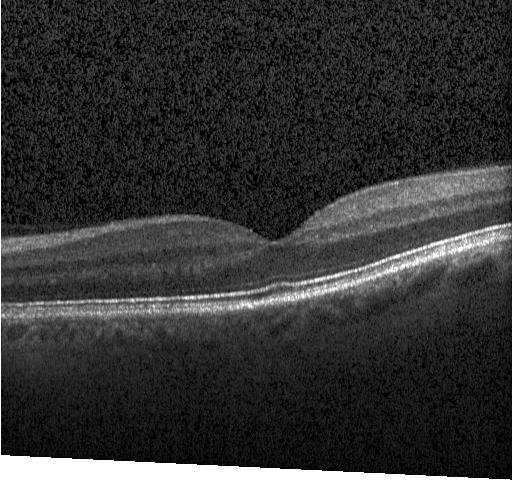 Heidelberg Spectralis OCT system. Retinal OCT B-scan. SD-OCT
Diagnosis: neither choroidal neovascularization, diabetic macular edema, nor drusen.